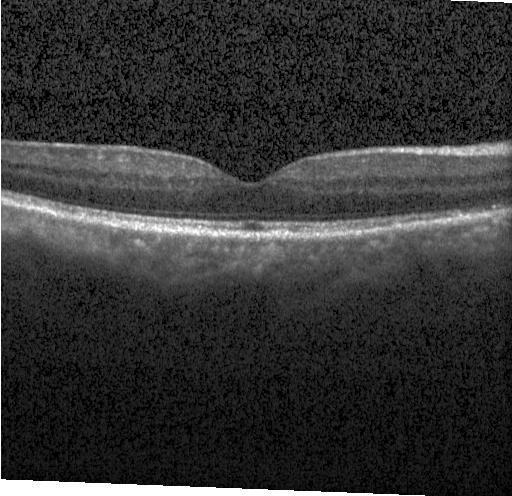 Heidelberg Spectralis OCT system; spectral-domain OCT; retinal OCT B-scan; horizontal scan through the fovea — Macular OCT: no evidence of choroidal neovascularization, diabetic macular edema, or drusen.